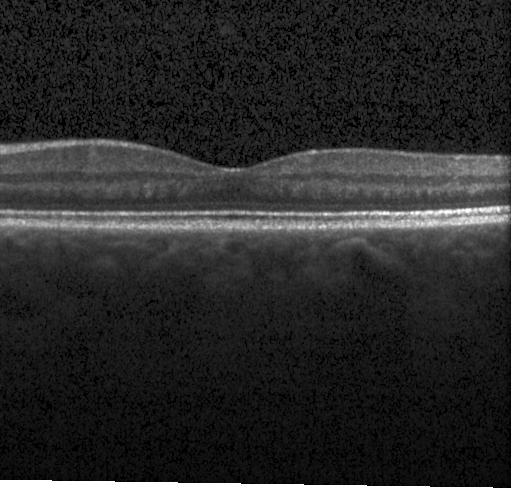
Impression: no CNV, DME, or drusen.